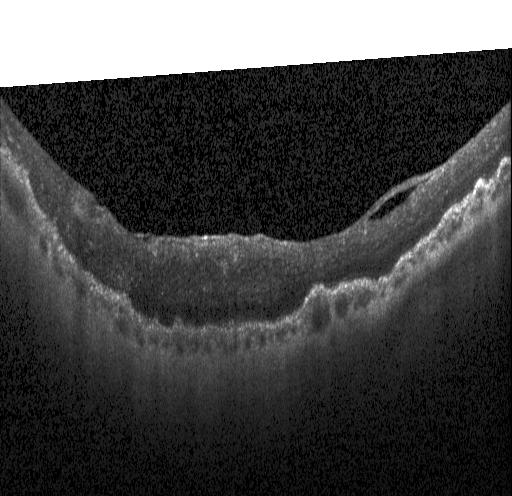 Through the macula · optical coherence tomography scan.
Dx: choroidal neovascularization.